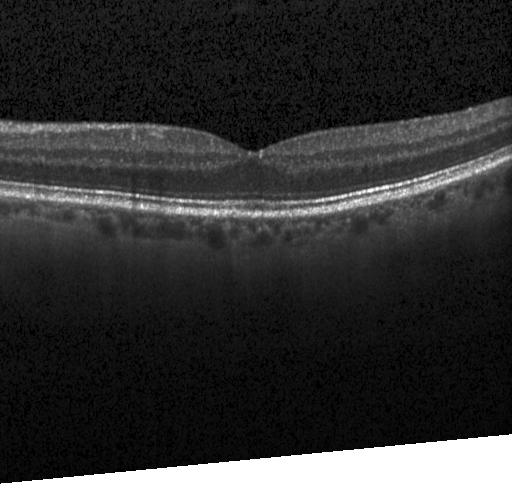

OCT B-scan showing no choroidal neovascularization, diabetic macular edema, or drusen.